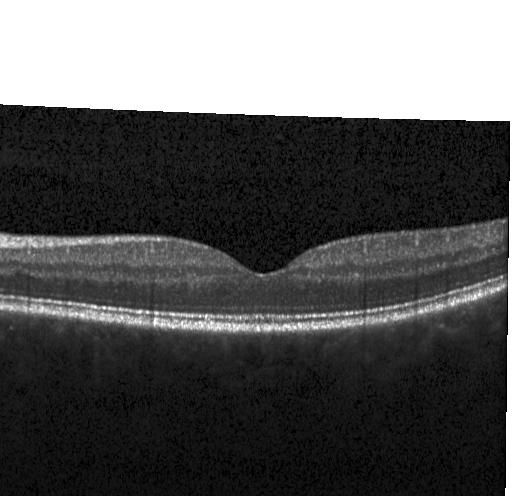

Retinal OCT cross-section showing neither CNV, DME, nor drusen.